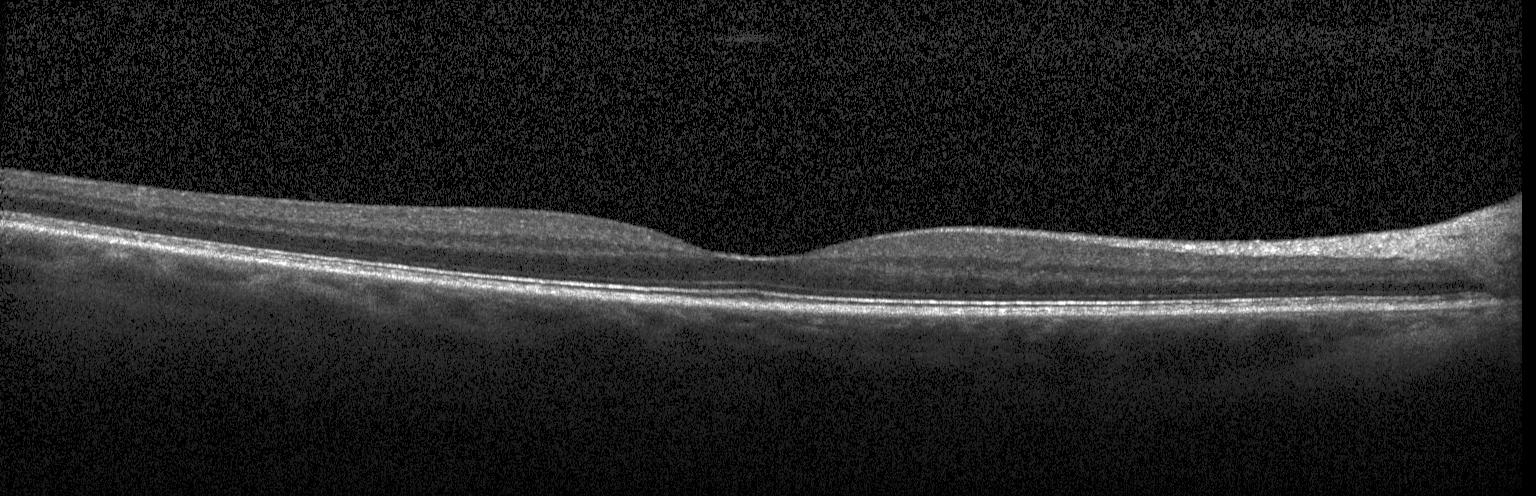 Spectral-domain OCT B-scan: no evidence of CNV, DME, or drusen.